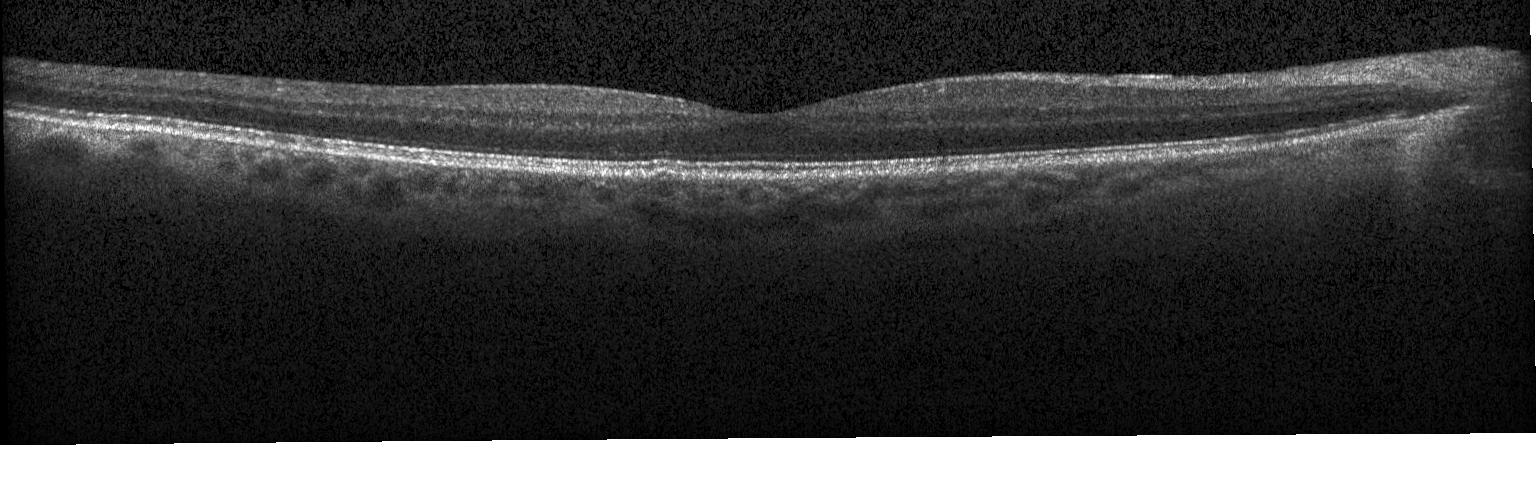 OCT finding: no evidence of CNV, DME, or drusen.